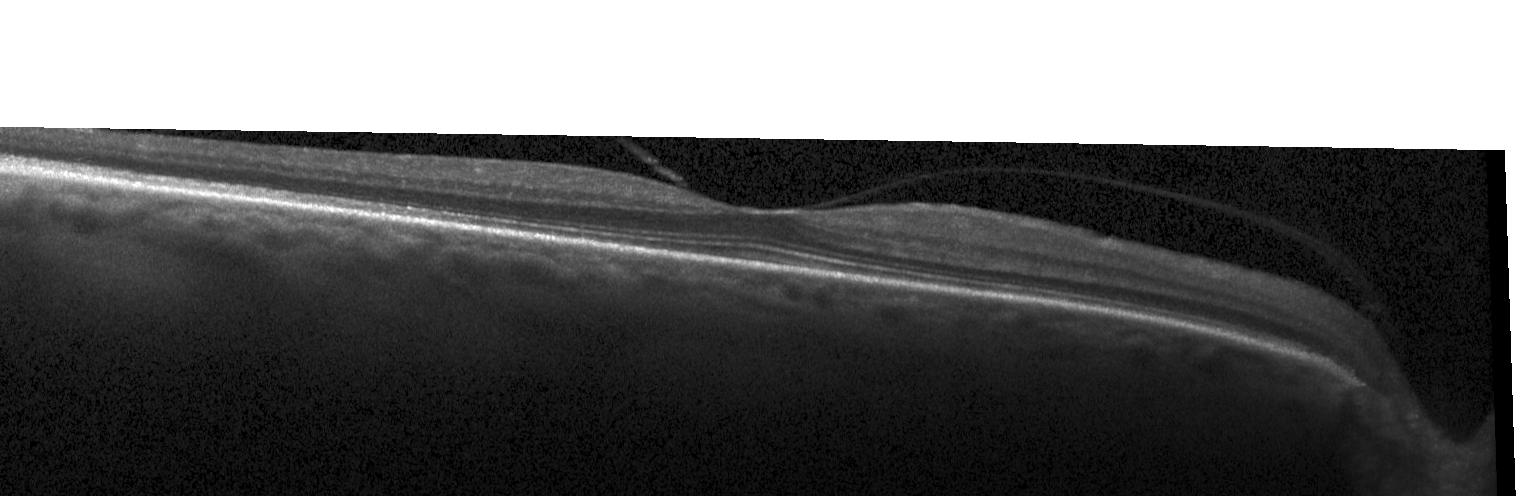

Spectral-domain optical coherence tomography. Optical coherence tomography B-scan — Finding: no choroidal neovascularization, no diabetic macular edema, and no drusen.